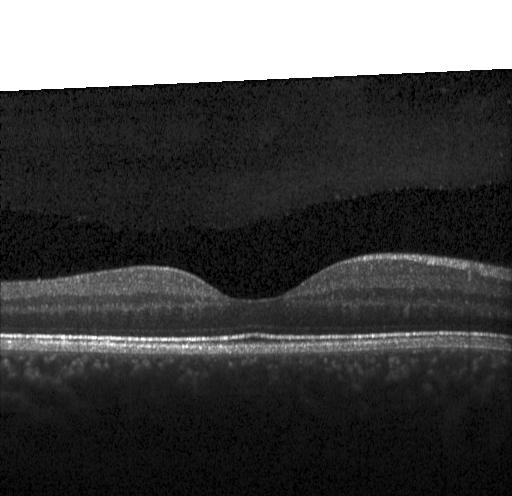 Centered on the fovea, instrument: Heidelberg Spectralis, optical coherence tomography scan.
Finding: no choroidal neovascularization, diabetic macular edema, or drusen.